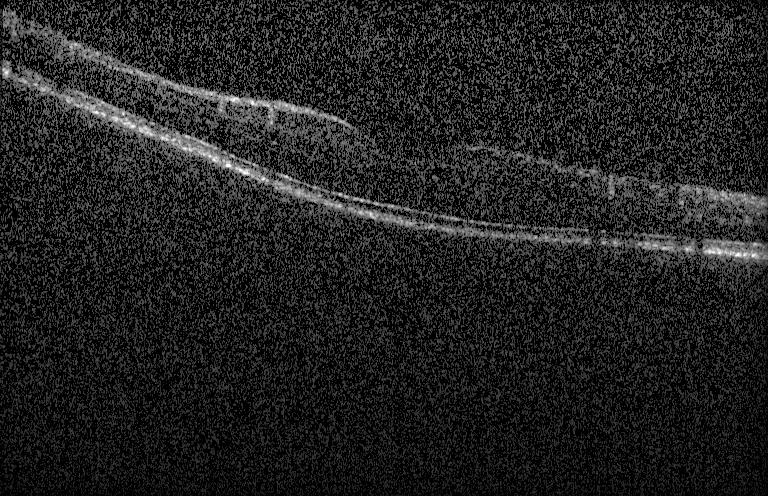
Retinal OCT cross-section showing no evidence of choroidal neovascularization, diabetic macular edema, or drusen.